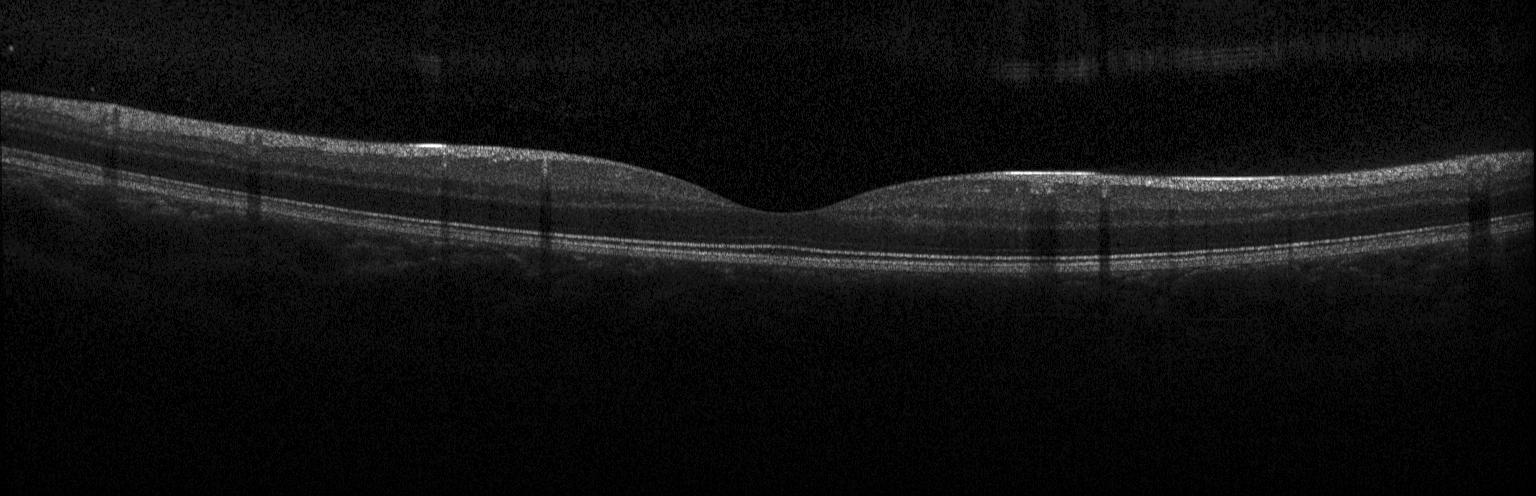

SD-OCT. OCT B-scan. Instrument: Heidelberg Spectralis
Dx: no choroidal neovascularization, diabetic macular edema, or drusen.